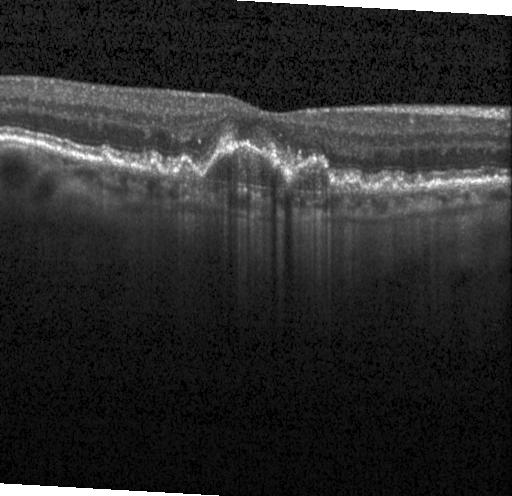

Spectral-domain OCT B-scan: a choroidal neovascular membrane.